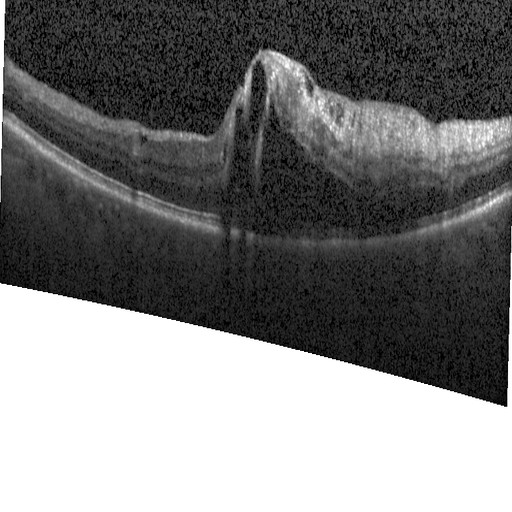
Through the macula · retinal OCT cross-section.
Diagnosis: diabetic macular edema.